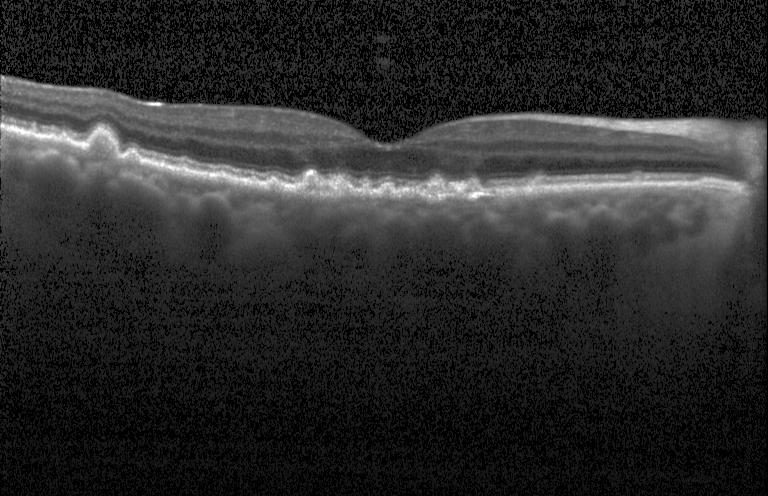

Macular scan. Spectral-domain optical coherence tomography. Retinal OCT B-scan. Heidelberg Spectralis — Assessment: sub-RPE drusenoid deposits.